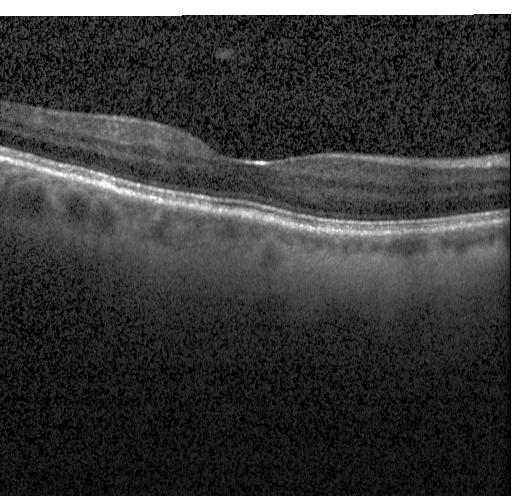
OCT line scan. Diagnosis: neither choroidal neovascularization, diabetic macular edema, nor drusen.